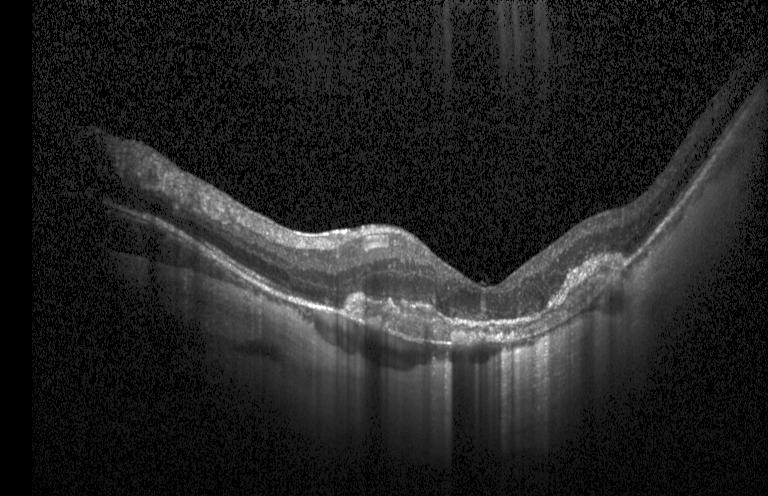
Optical coherence tomography B-scan
Impression: choroidal neovascularization.